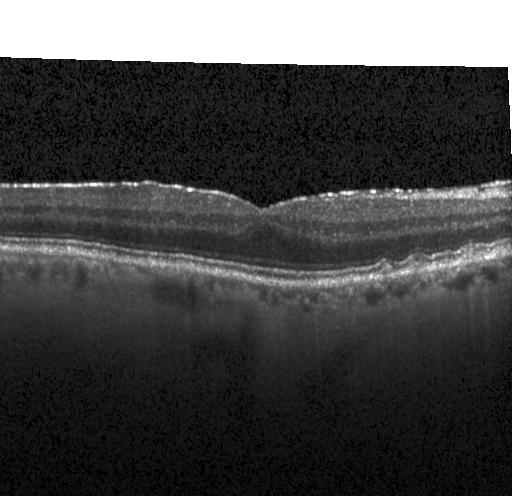 Diagnosis: drusen.